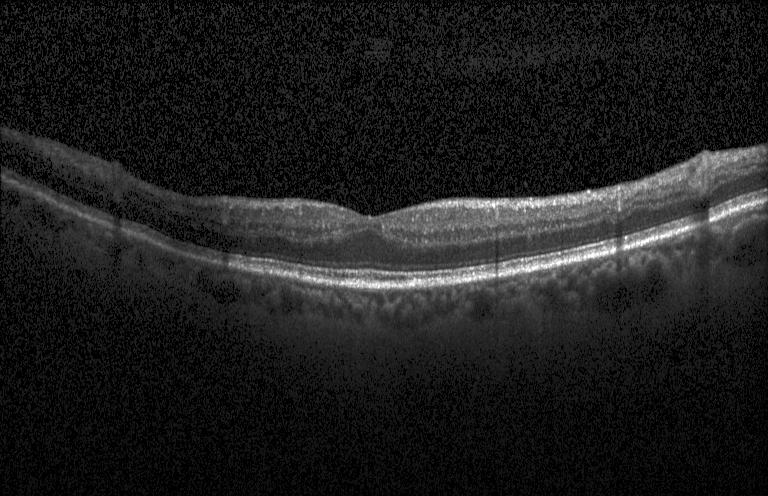 Spectral-domain OCT. Optical coherence tomography B-scan. OCT finding: neither choroidal neovascularization, diabetic macular edema, nor drusen.